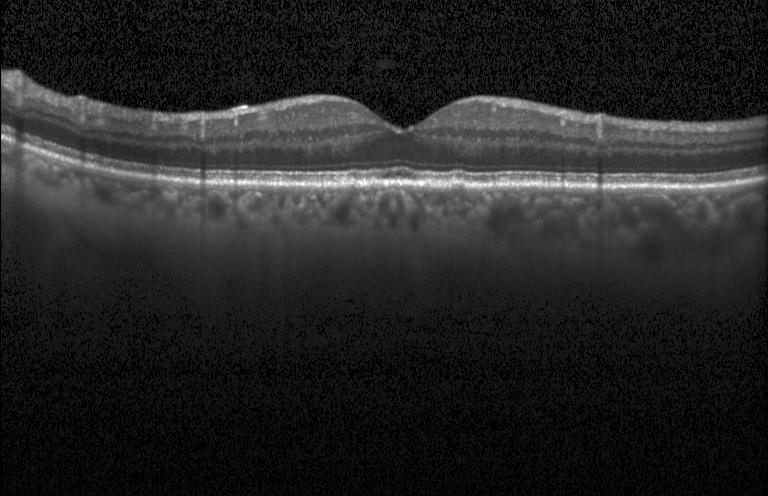
Spectral-domain optical coherence tomography. Fovea-centered. Retinal OCT B-scan.
Dx: no choroidal neovascularization, diabetic macular edema, or drusen.